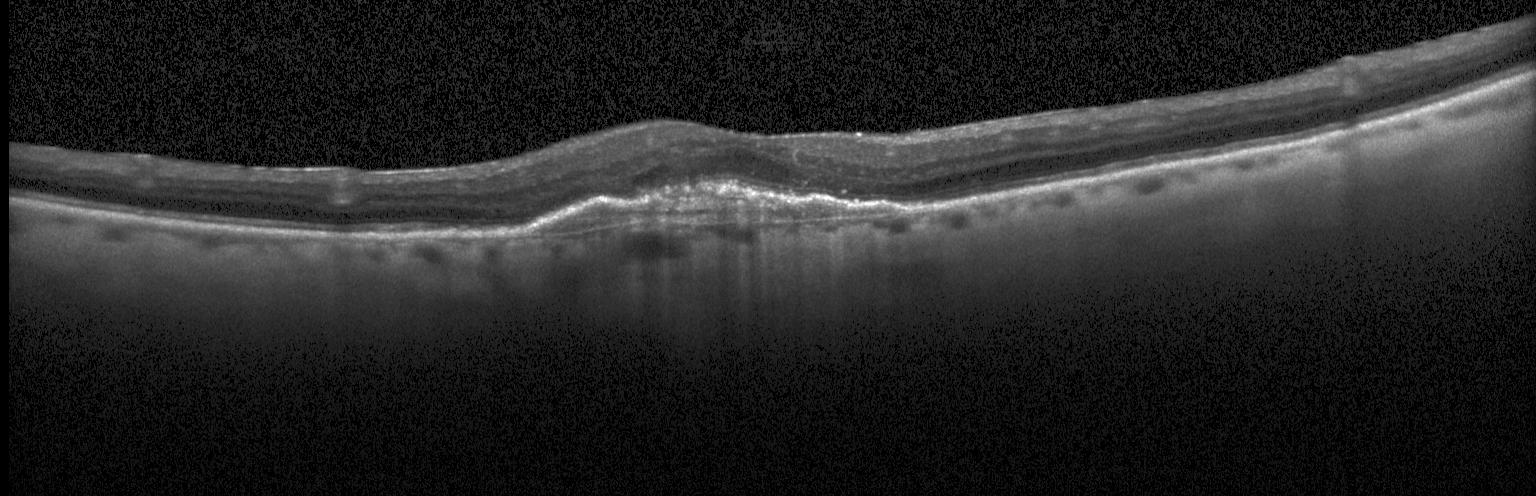 Dx: a choroidal neovascular membrane.